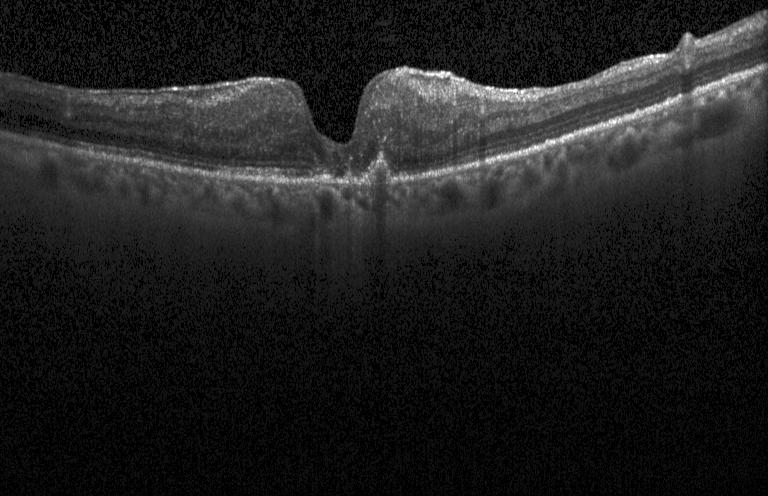

OCT line scan · acquired on a Heidelberg Spectralis · spectral-domain optical coherence tomography — Dx: CNV.